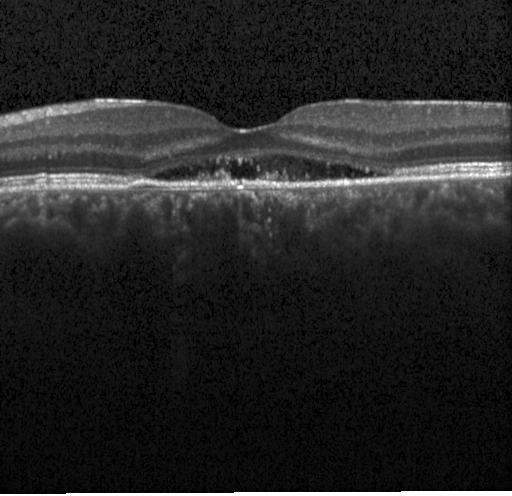

Retinal OCT cross-section · acquired on a Heidelberg Spectralis · macular scan.
OCT finding: a choroidal neovascular membrane.